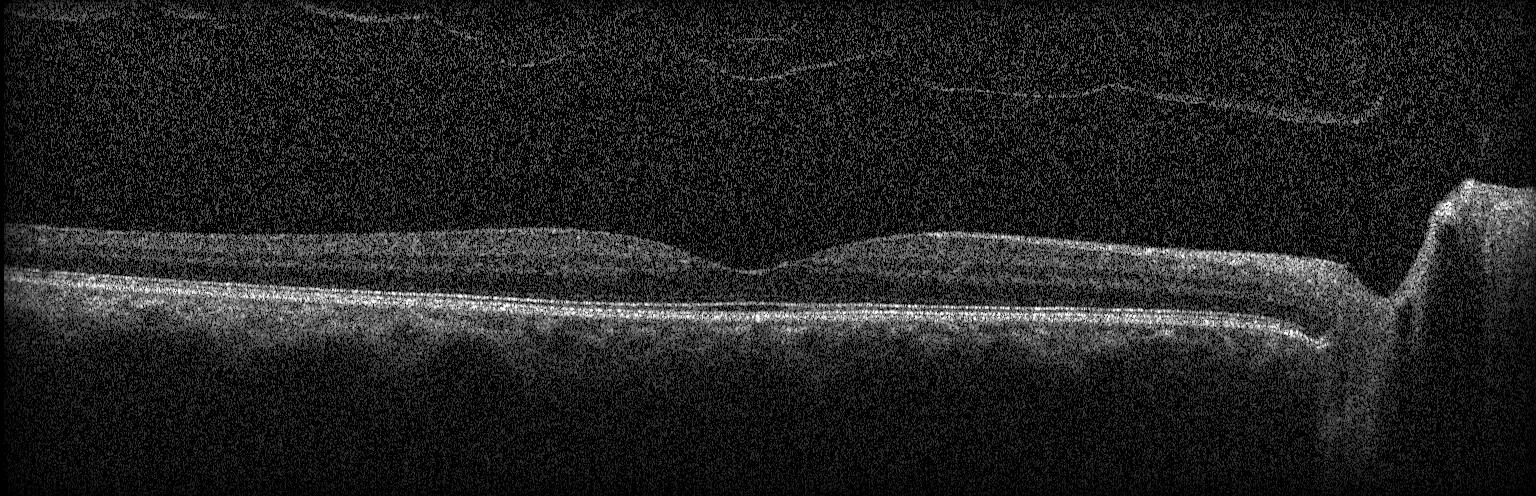 Finding: no choroidal neovascularization, diabetic macular edema, or drusen.